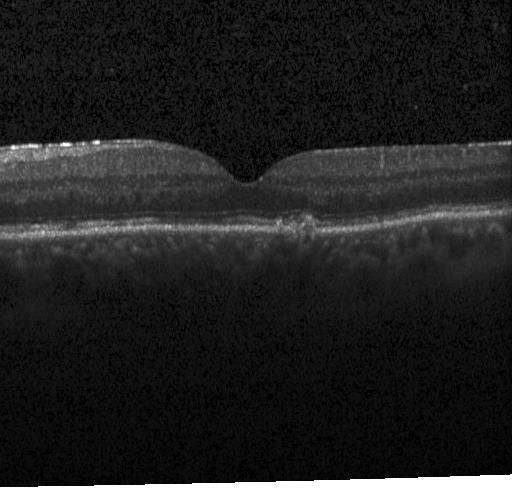 Fovea-centered · optical coherence tomography B-scan · spectral-domain optical coherence tomography.
This B-scan demonstrates drusen.